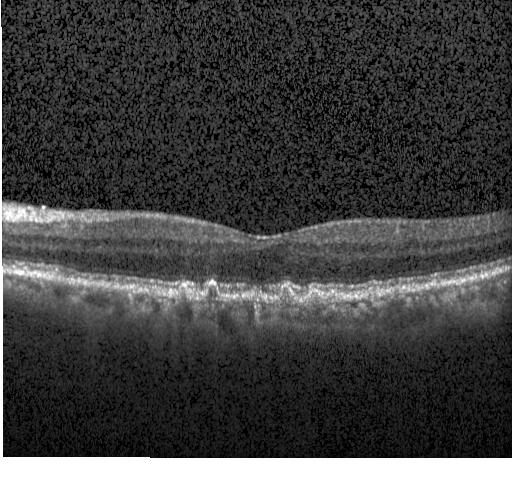 Finding: drusen.